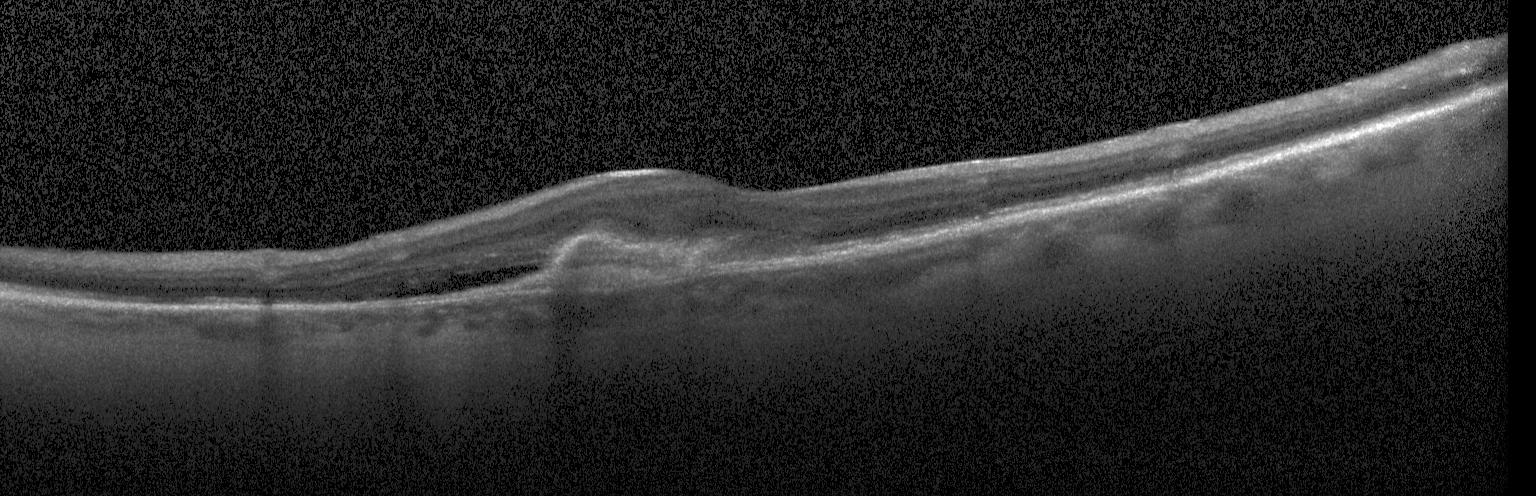 Instrument: Heidelberg Spectralis · OCT B-scan · spectral-domain optical coherence tomography.
OCT finding: choroidal neovascularization.